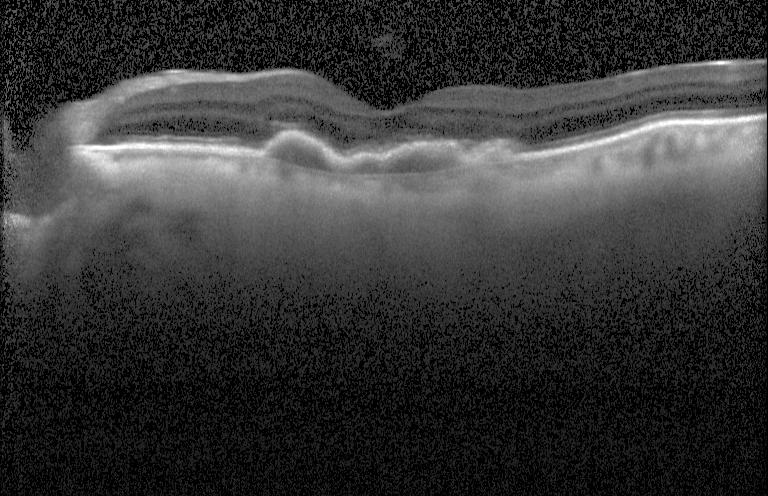
Optical coherence tomography B-scan, fovea-centered, acquired on a Heidelberg Spectralis — The scan shows CNV.